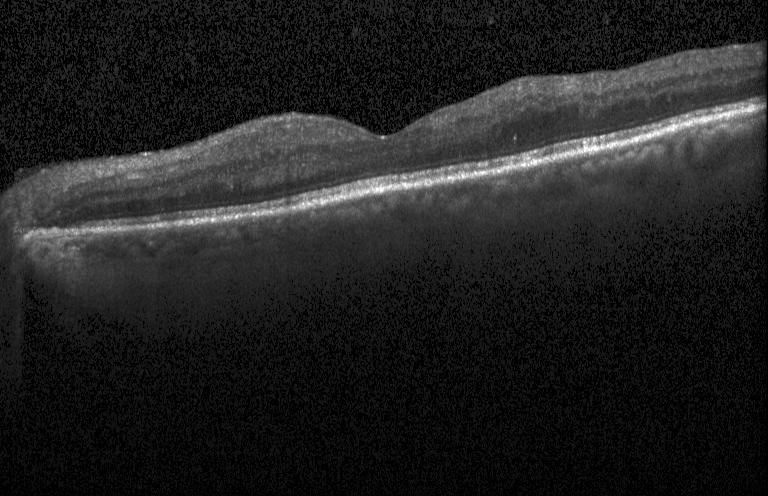
Retinal OCT cross-section — Assessment: no CNV, no DME, and no drusen.